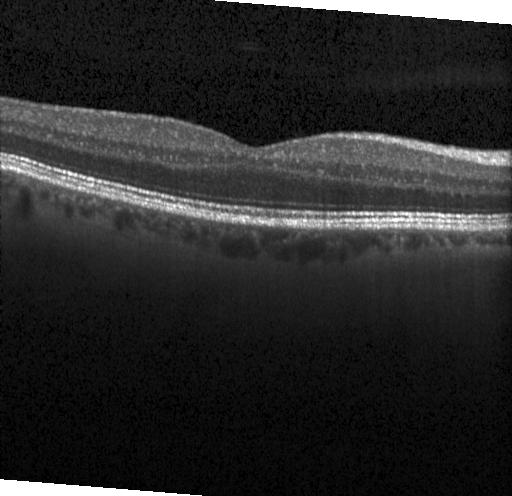

OCT line scan.
Impression: no choroidal neovascularization, no diabetic macular edema, and no drusen.